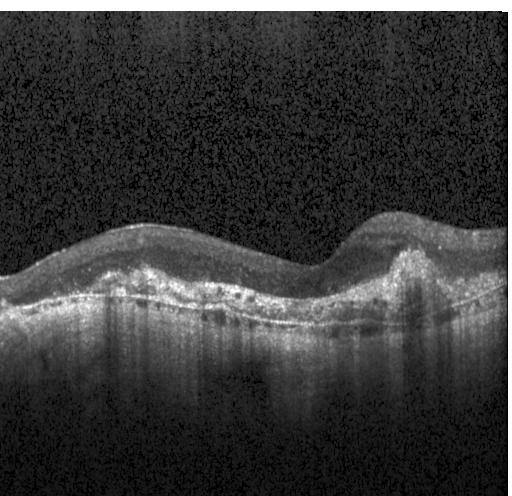

Optical coherence tomography B-scan — Diagnosis: choroidal neovascularization (CNV).